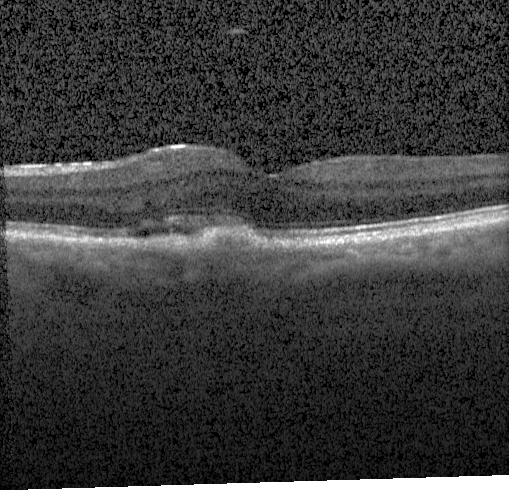

Fovea-centered · OCT B-scan.
Diagnosis: a choroidal neovascular membrane.